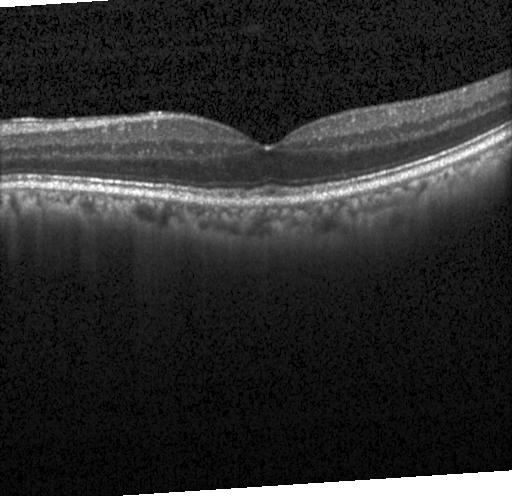

Retinal OCT cross-section · instrument: Heidelberg Spectralis · spectral-domain optical coherence tomography · through the macula
Diagnosis: no CNV, no DME, and no drusen.